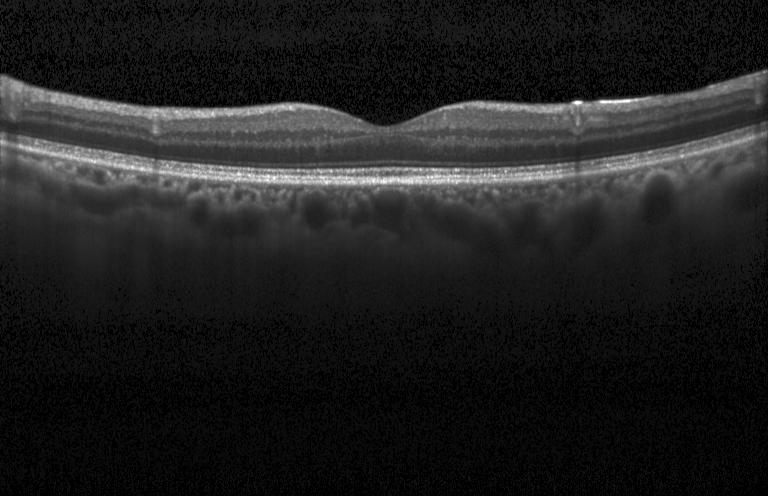 Macular scan; spectral-domain optical coherence tomography; OCT line scan; Heidelberg Spectralis OCT system
Assessment: no choroidal neovascularization, diabetic macular edema, or drusen.